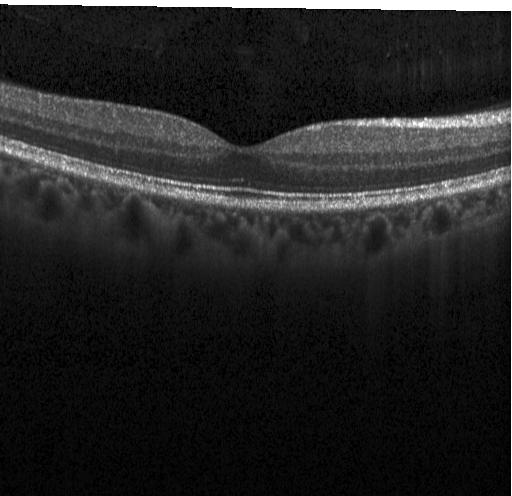 OCT B-scan
Diagnosis: no CNV, DME, or drusen.